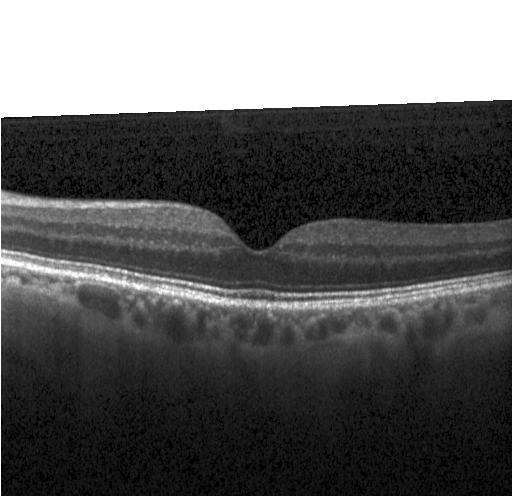 OCT line scan. Impression: no evidence of CNV, DME, or drusen.